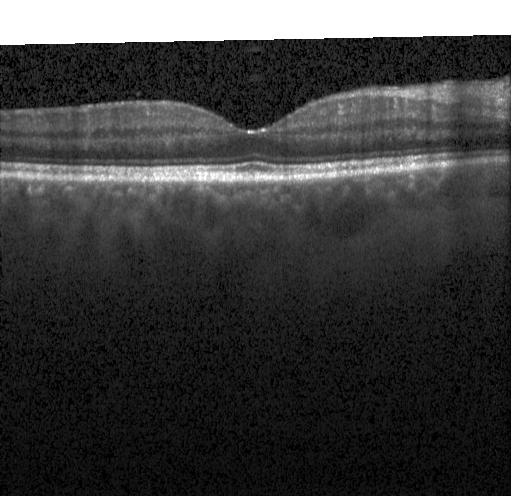

OCT line scan — The scan shows no evidence of choroidal neovascularization, diabetic macular edema, or drusen.